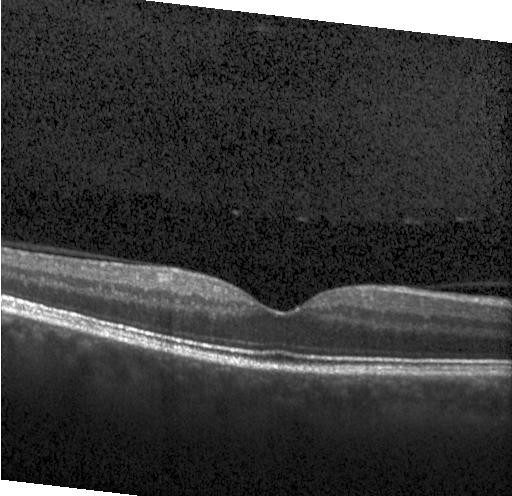 This B-scan demonstrates no choroidal neovascularization, diabetic macular edema, or drusen.